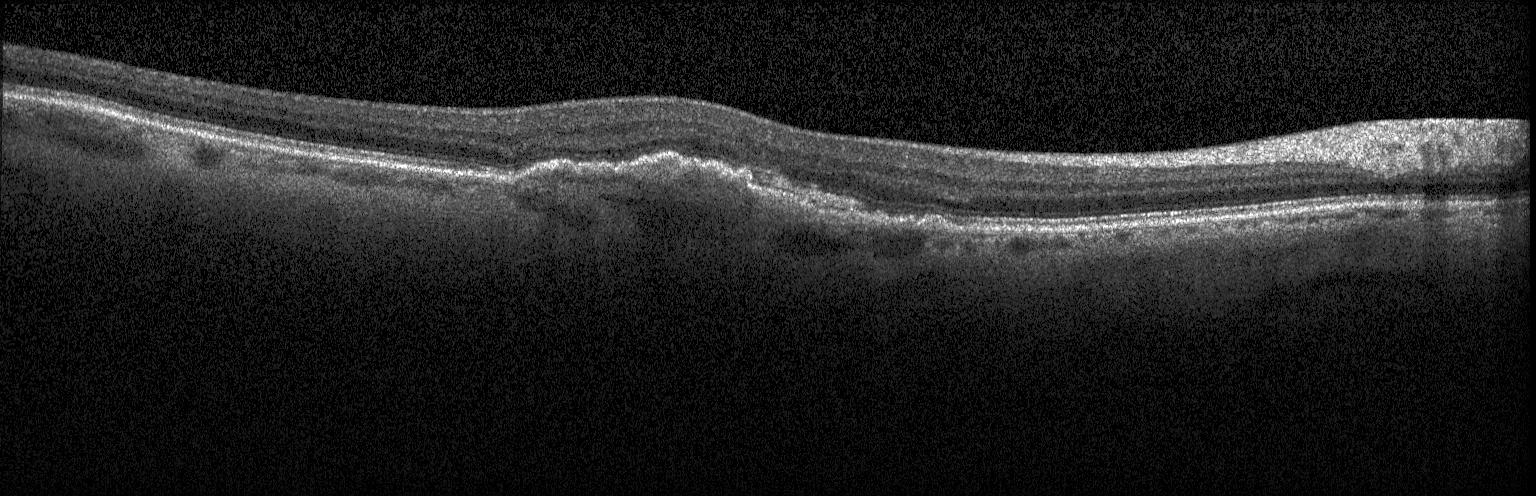
SD-OCT · through the macula · Heidelberg Spectralis · optical coherence tomography B-scan — This B-scan demonstrates CNV.